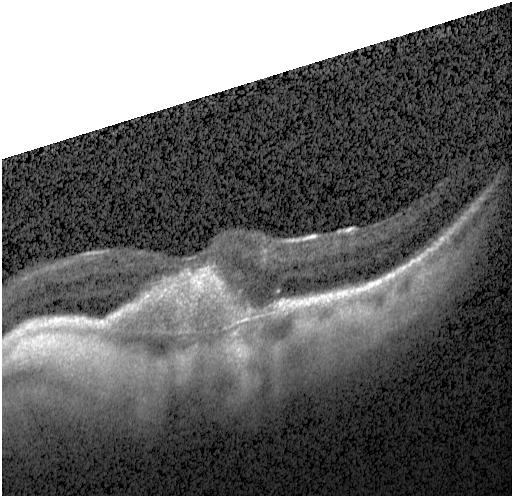

Retinal OCT B-scan; instrument: Heidelberg Spectralis — Finding: choroidal neovascularization (CNV).